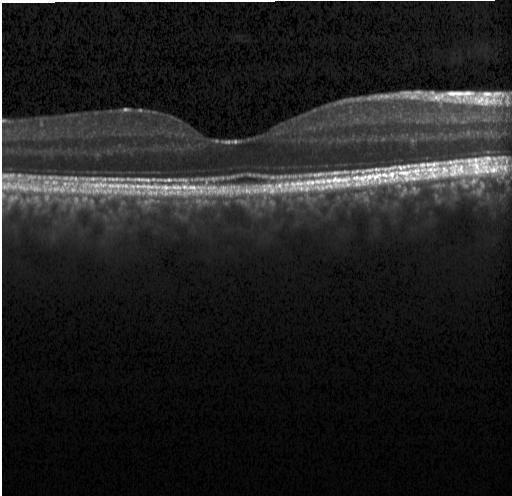
Fovea-centered; optical coherence tomography B-scan — No choroidal neovascularization, no diabetic macular edema, and no drusen.